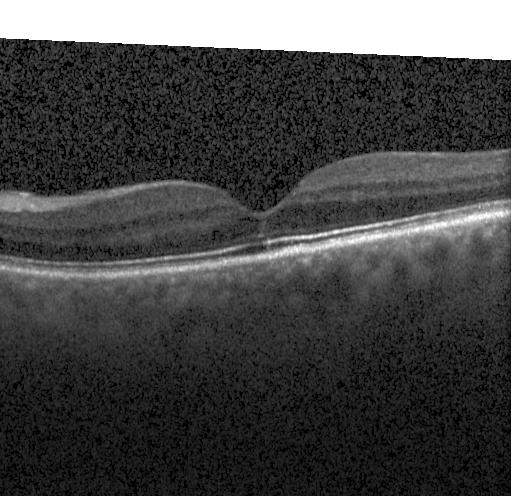
Macular OCT: no choroidal neovascularization, no diabetic macular edema, and no drusen.